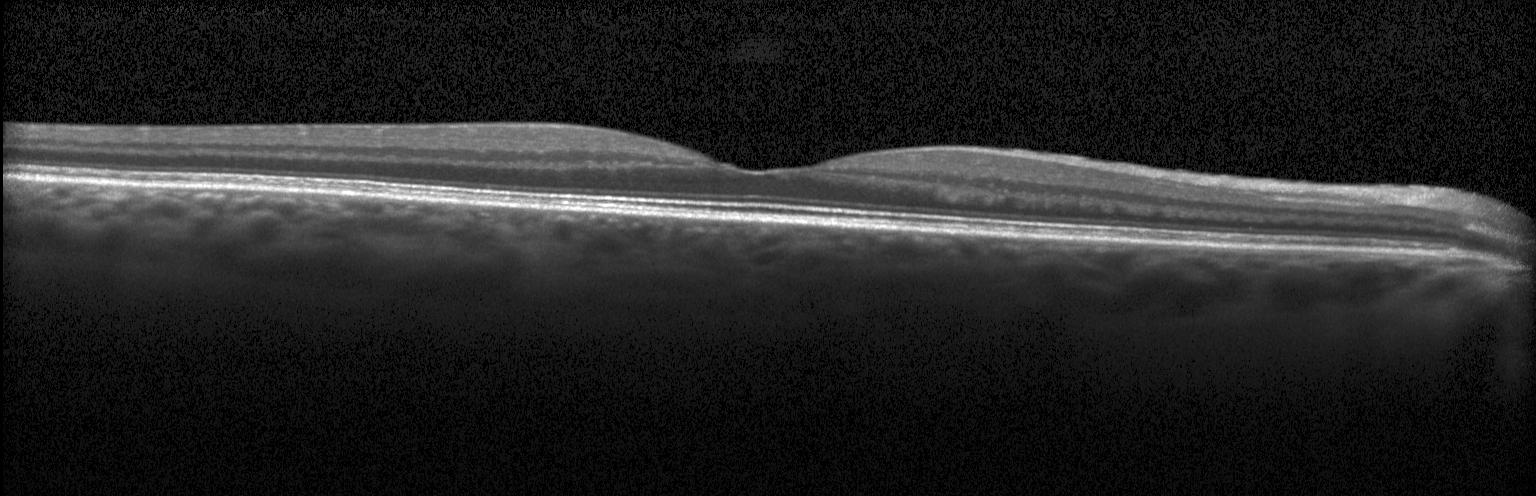

Acquired on a Heidelberg Spectralis; optical coherence tomography B-scan
Impression: neither choroidal neovascularization, diabetic macular edema, nor drusen.